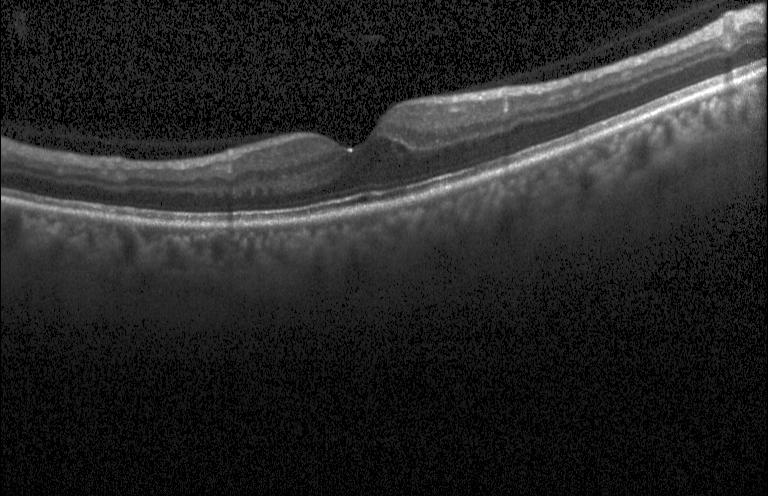
OCT B-scan.
The scan shows no evidence of CNV, DME, or drusen.